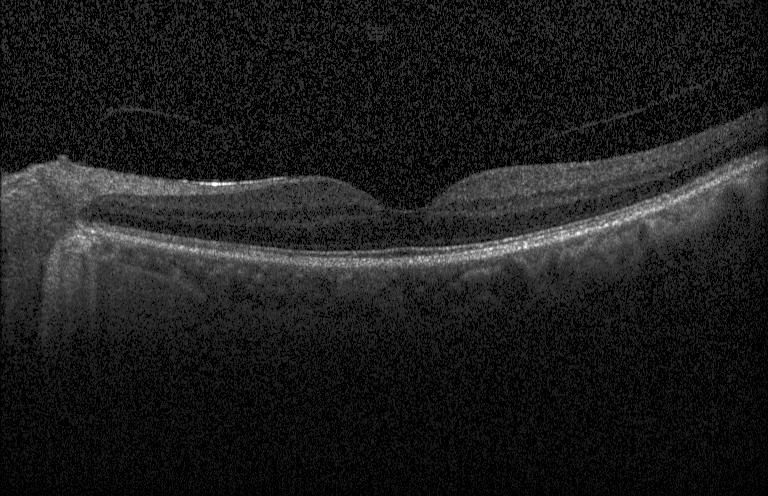 OCT B-scan showing neither choroidal neovascularization, diabetic macular edema, nor drusen.